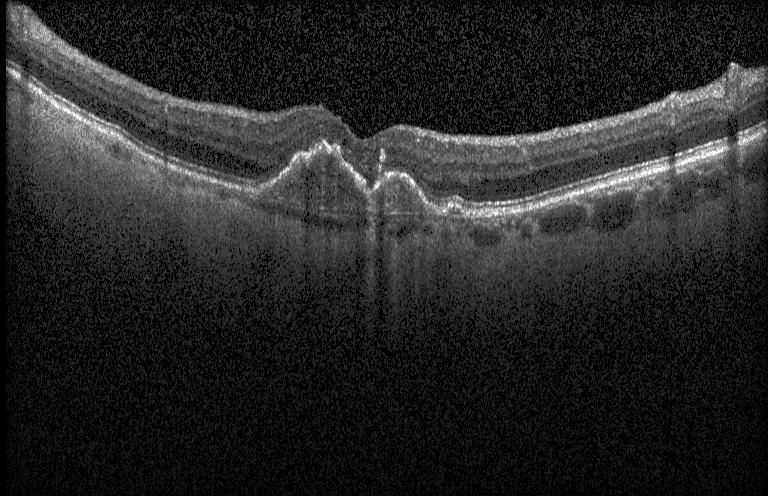

Finding: CNV.